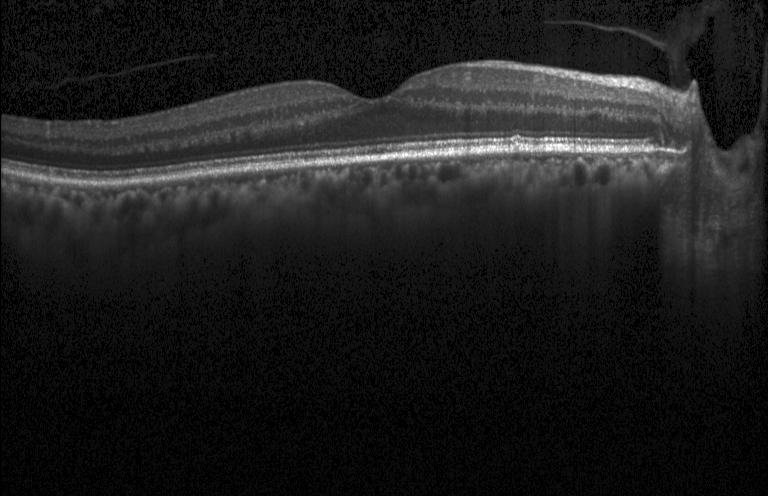 Macular OCT: no evidence of choroidal neovascularization, diabetic macular edema, or drusen.